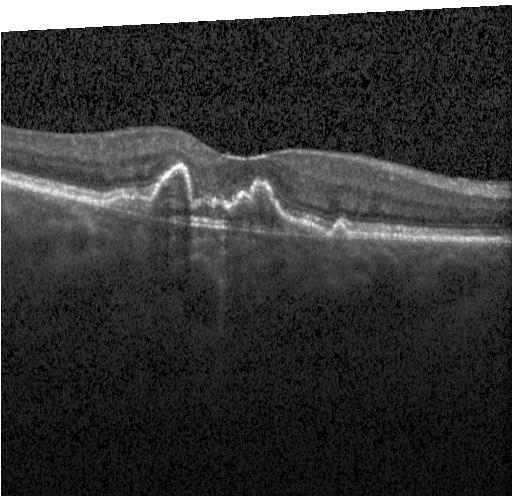 Assessment: CNV.